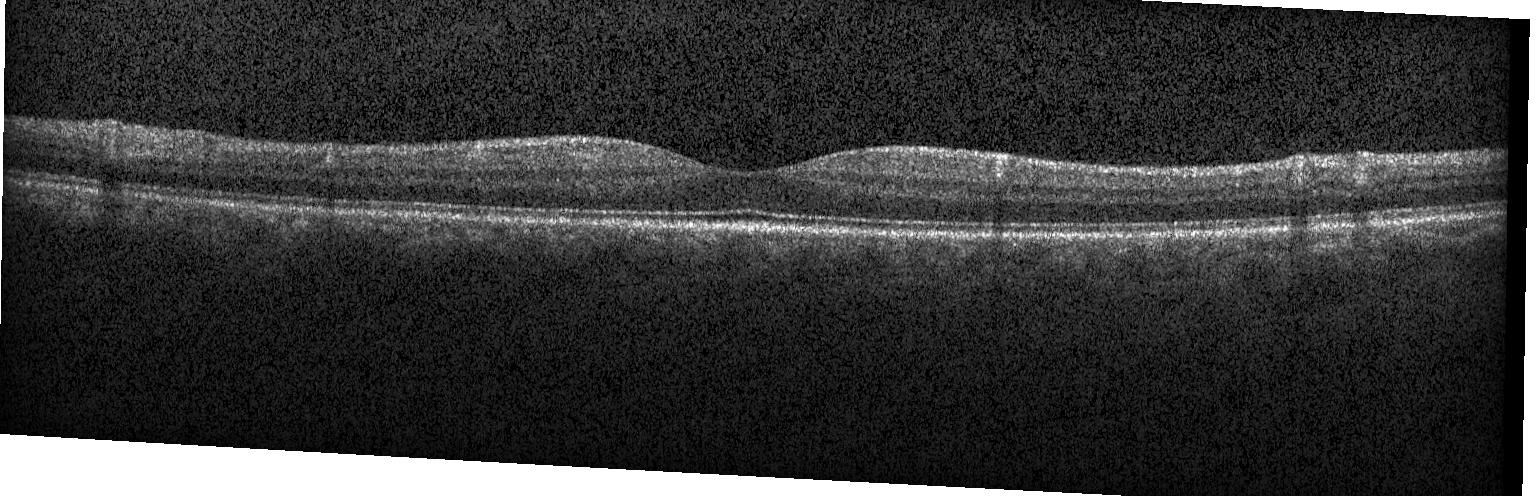 Optical coherence tomography B-scan — Impression: no evidence of choroidal neovascularization, diabetic macular edema, or drusen.